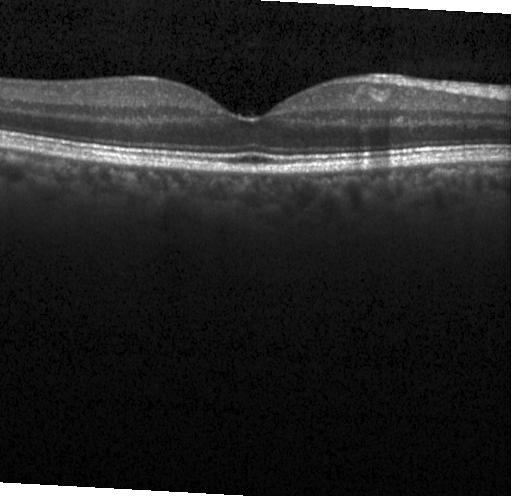
Optical coherence tomography scan
Finding: no choroidal neovascularization, diabetic macular edema, or drusen.